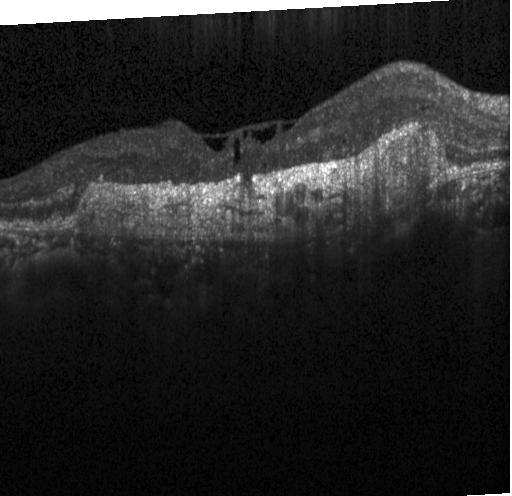 Spectral-domain OCT B-scan: CNV.